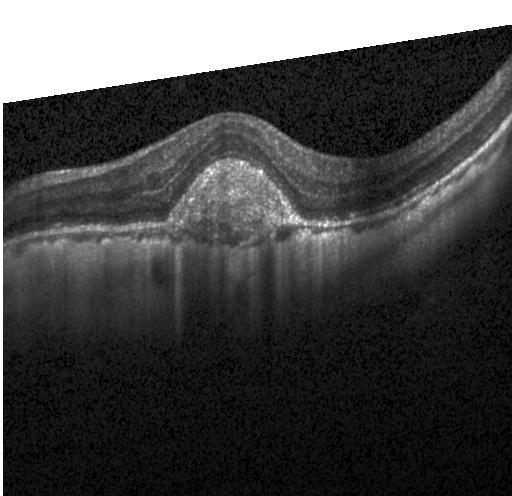 Macular OCT demonstrating CNV.